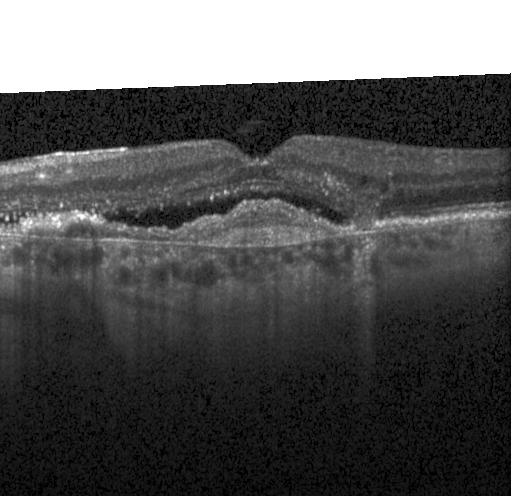
Macular OCT: CNV.